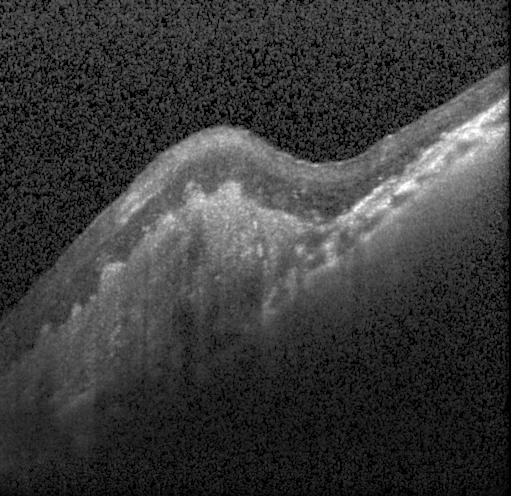 Optical coherence tomography B-scan · through the macula · spectral-domain optical coherence tomography.
This B-scan demonstrates a choroidal neovascular membrane.